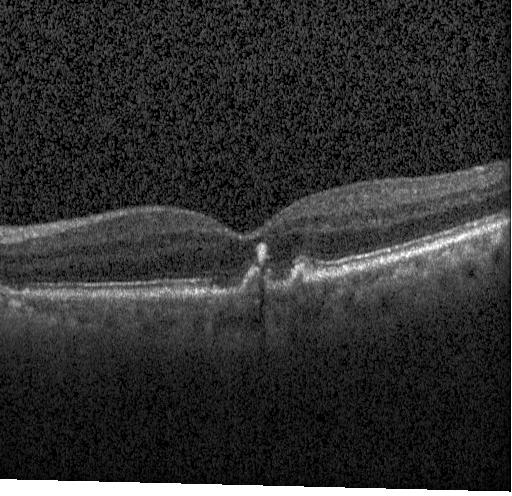
Retinal OCT cross-section.
Dx: multiple drusen.